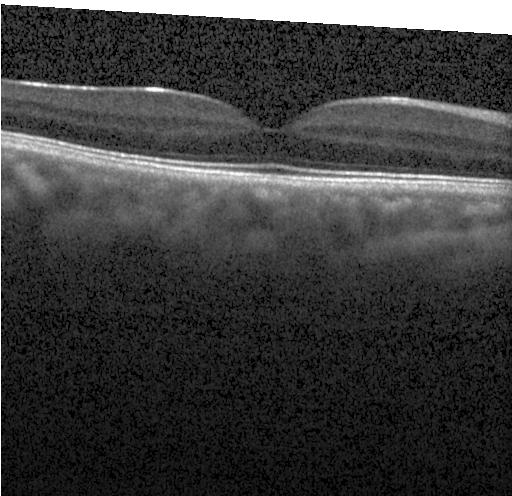
OCT line scan, horizontal scan through the fovea, spectral-domain OCT, instrument: Heidelberg Spectralis — The scan shows no CNV, DME, or drusen.